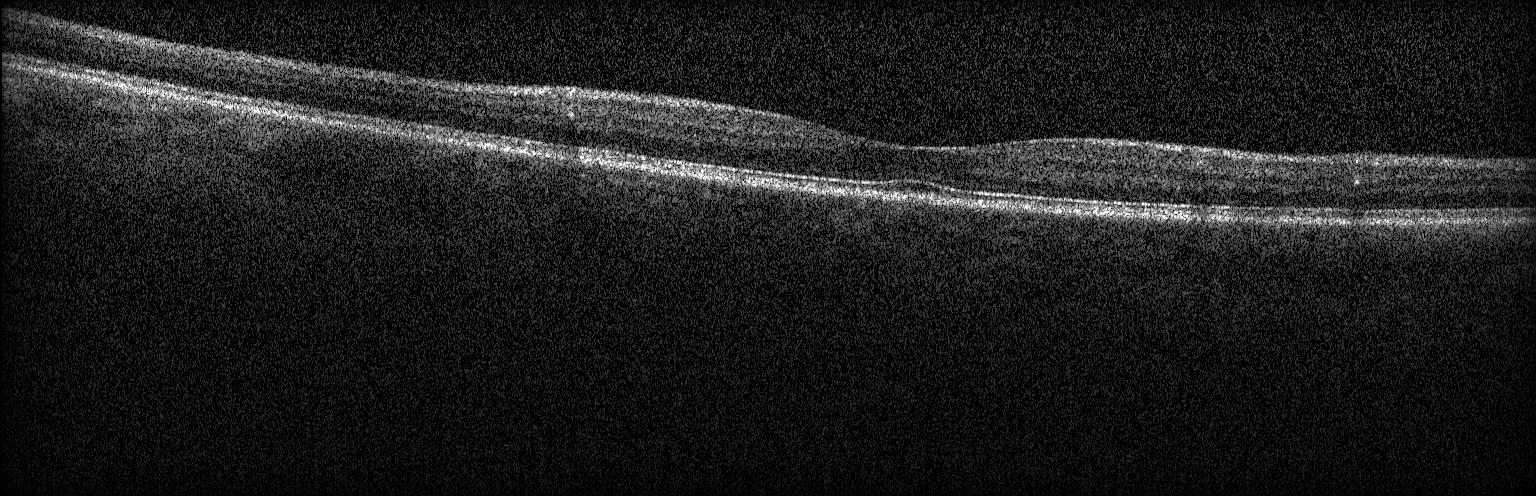 Optical coherence tomography B-scan
No choroidal neovascularization, no diabetic macular edema, and no drusen.